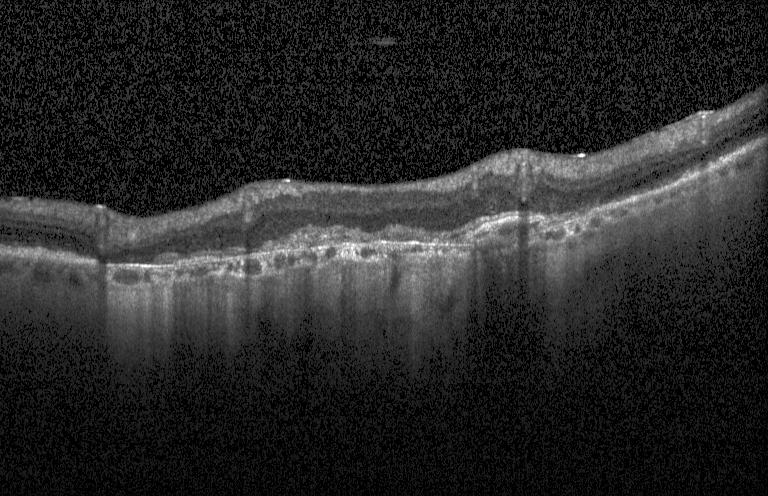
Acquired on a Heidelberg Spectralis. OCT line scan. Spectral-domain OCT. Centered on the fovea. Dx: a choroidal neovascular membrane.